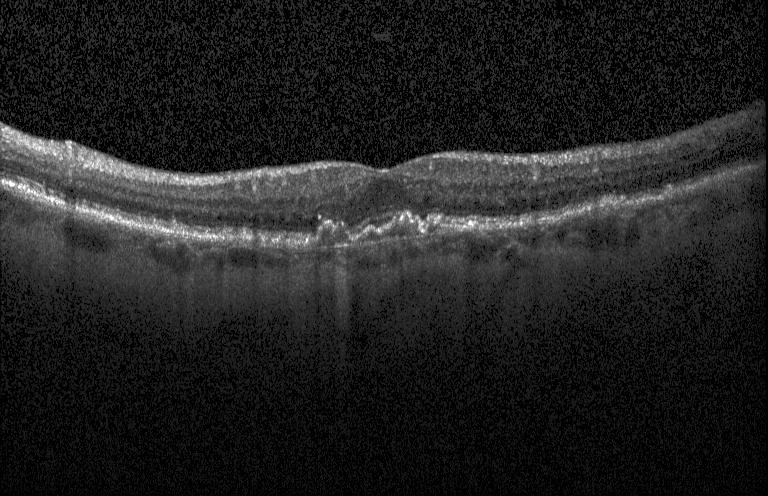

Impression: CNV.